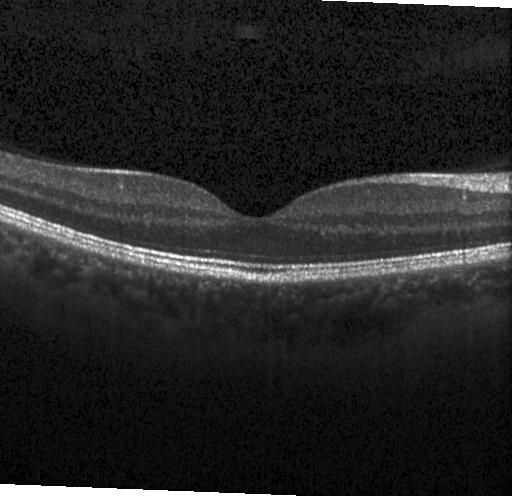 OCT B-scan, Heidelberg Spectralis OCT system, spectral-domain OCT.
Dx: no choroidal neovascularization, diabetic macular edema, or drusen.